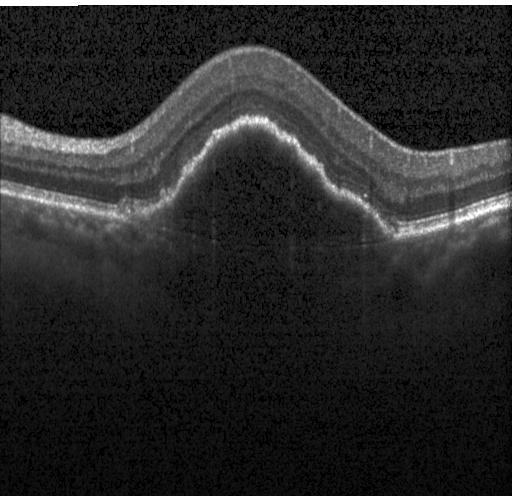

Finding: choroidal neovascularization (CNV).